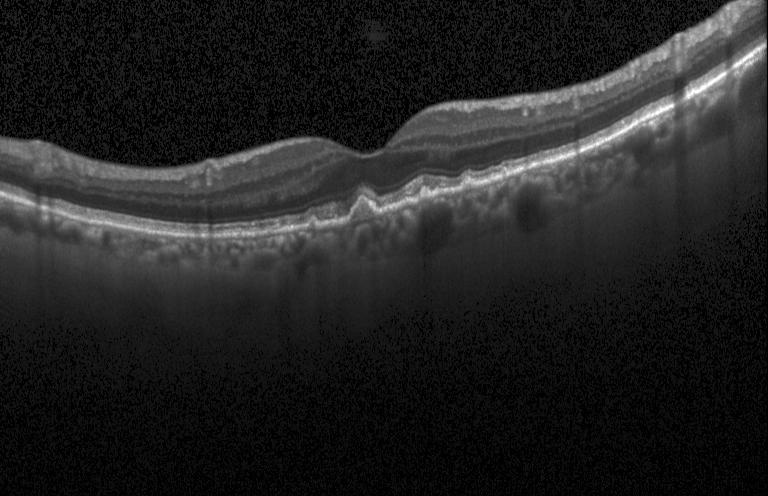 Macular OCT demonstrating sub-RPE drusenoid deposits.